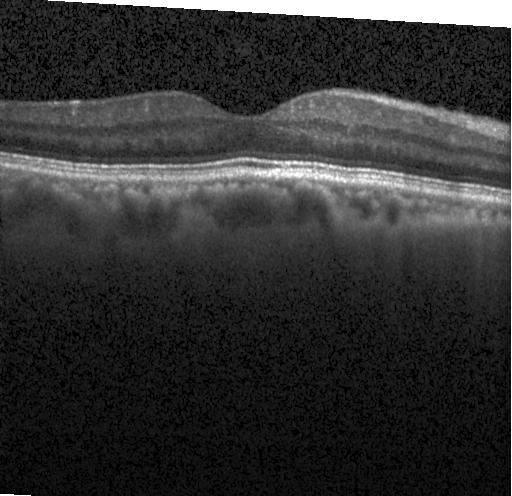
Optical coherence tomography B-scan, Heidelberg Spectralis, horizontal scan through the fovea, SD-OCT.
Assessment: neither choroidal neovascularization, diabetic macular edema, nor drusen.